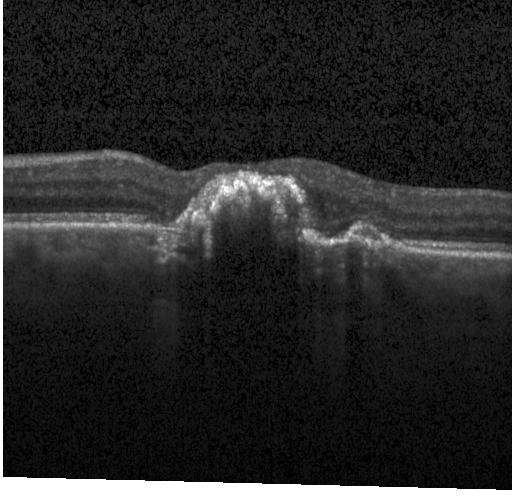
Spectral-domain OCT · instrument: Heidelberg Spectralis · retinal OCT B-scan · through the macula
Assessment: a choroidal neovascular membrane.